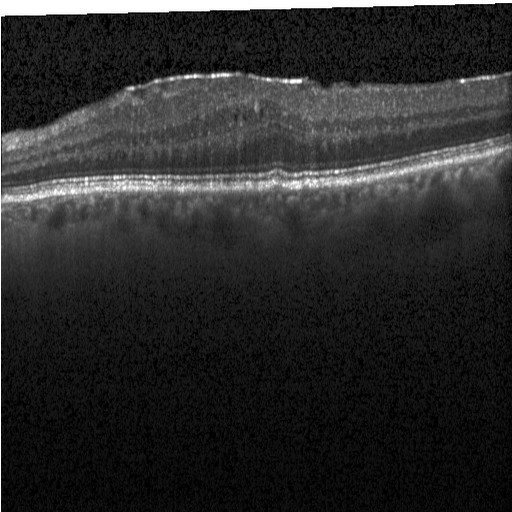
SD-OCT · retinal OCT B-scan · Heidelberg Spectralis OCT system · horizontal scan through the fovea
Impression: DME.